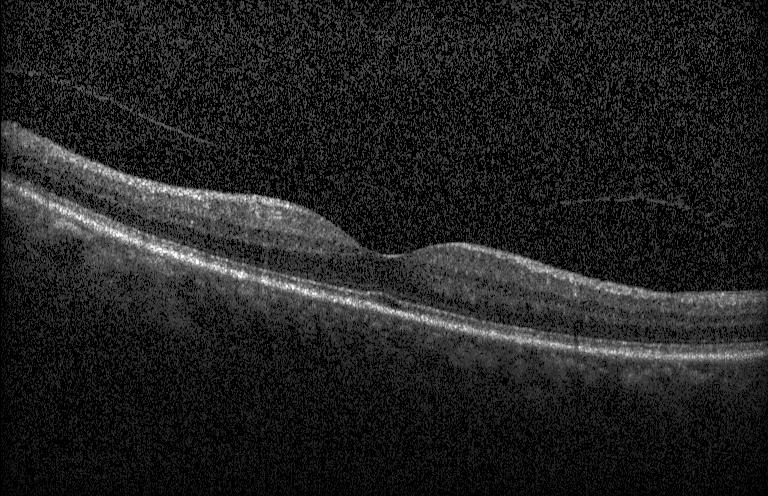

OCT B-scan. Impression: no evidence of choroidal neovascularization, diabetic macular edema, or drusen.